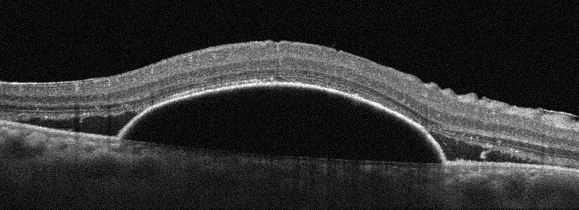

Optovue Avanti RTVue XR; macular scan; OD; retinal OCT B-scan — Age-related macular degeneration.